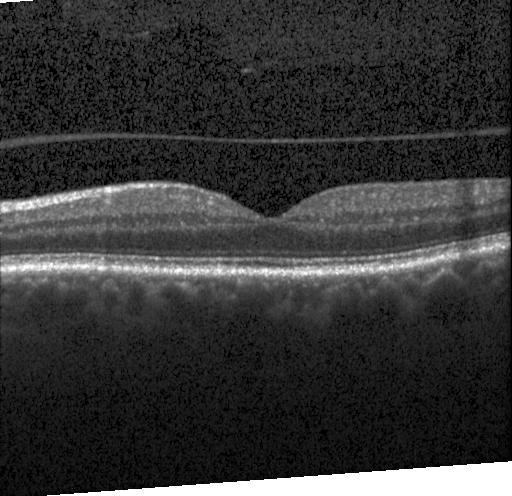 OCT finding: no choroidal neovascularization, diabetic macular edema, or drusen.